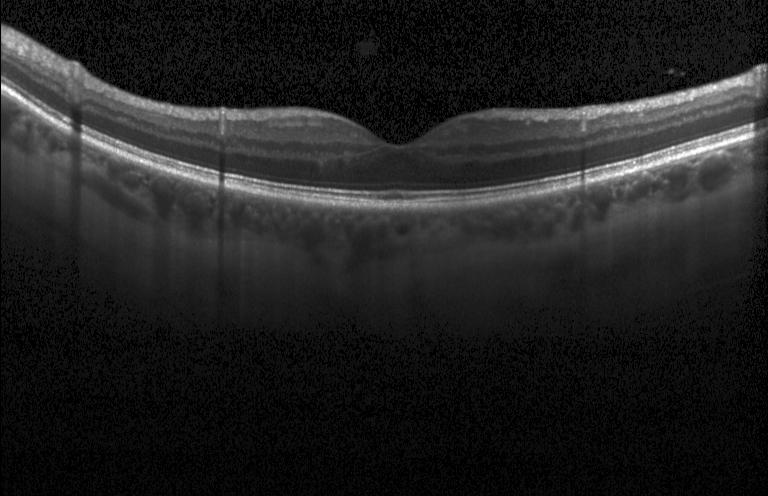

OCT B-scan showing neither CNV, DME, nor drusen.